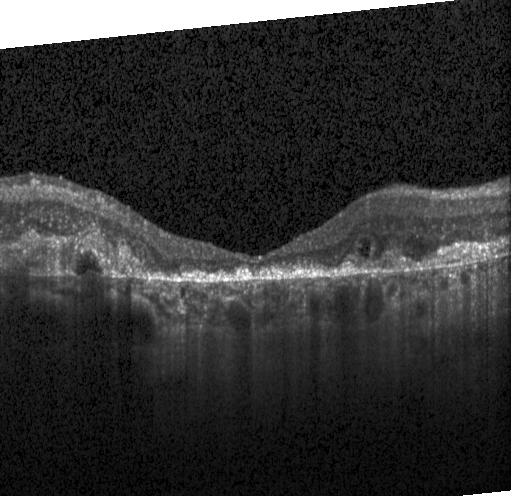

Optical coherence tomography scan; through the macula
OCT finding: choroidal neovascularization (CNV).